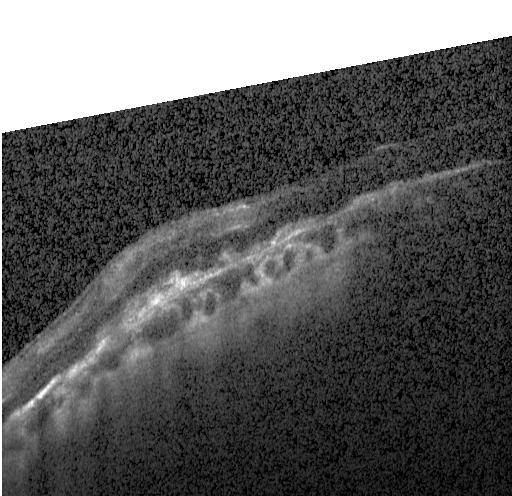

Retinal OCT cross-section · spectral-domain OCT. Dx: a choroidal neovascular membrane.